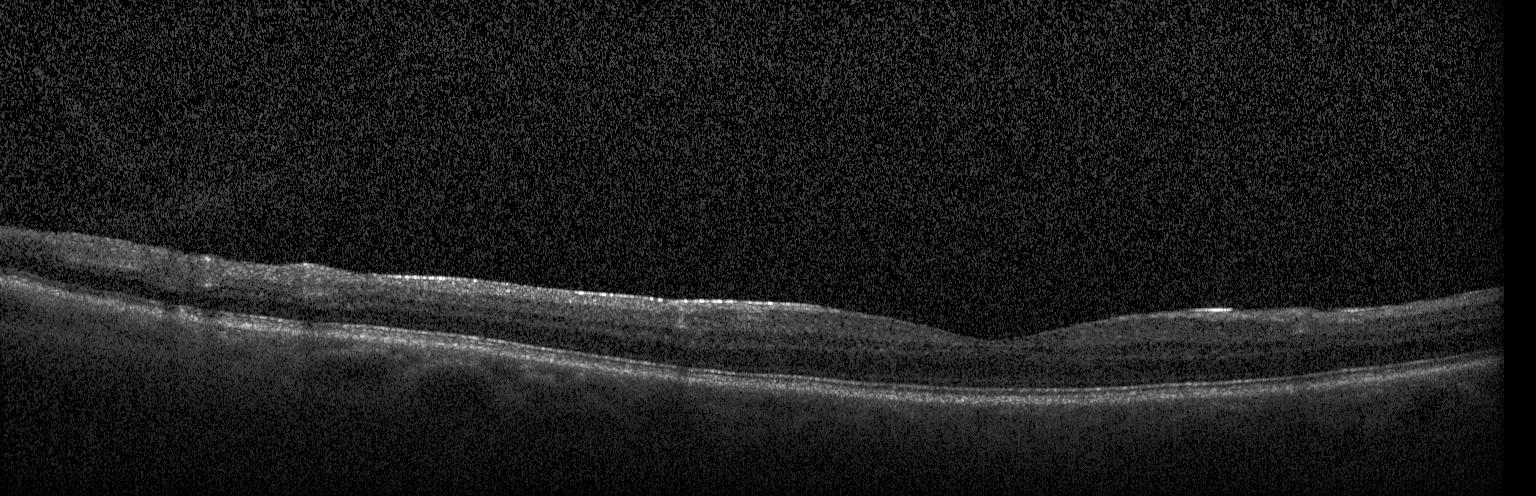 Macular OCT demonstrating no choroidal neovascularization, no diabetic macular edema, and no drusen.